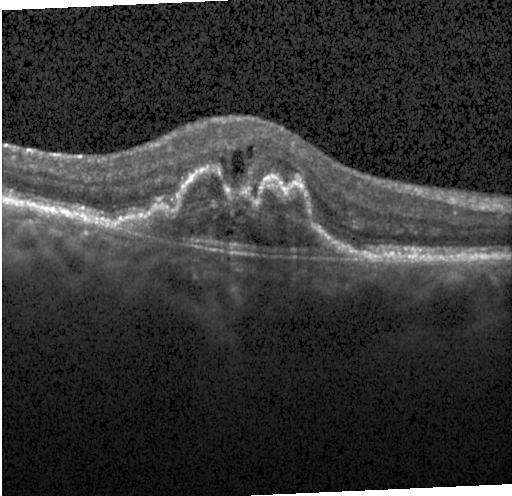 Impression: a choroidal neovascular membrane.